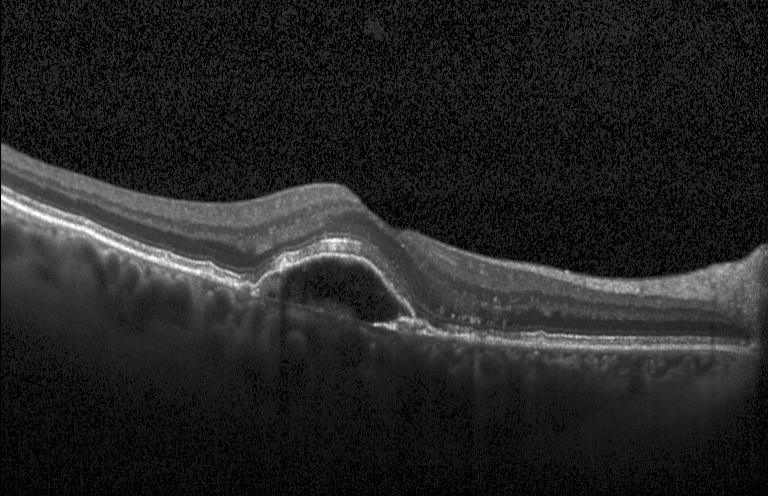 OCT B-scan showing CNV.